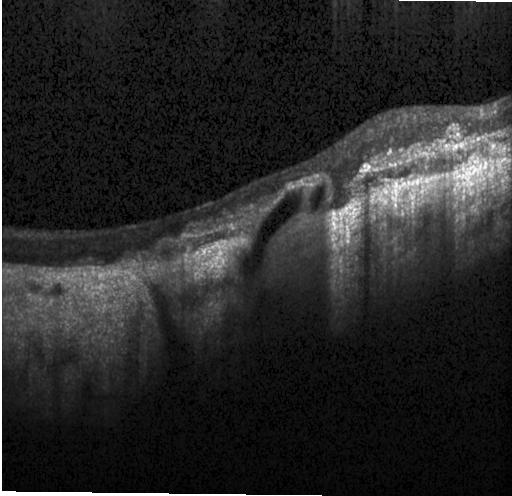 Retinal OCT cross-section showing CNV.